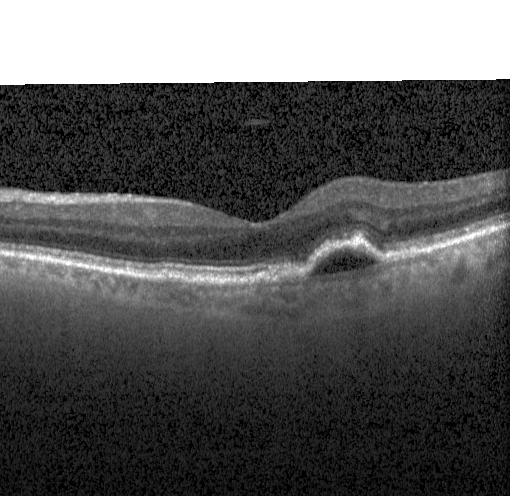

OCT line scan. OCT finding: choroidal neovascularization (CNV).